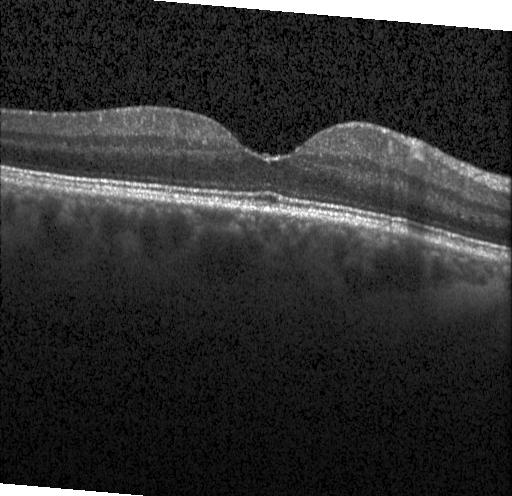 Optical coherence tomography B-scan — Macular OCT: no evidence of choroidal neovascularization, diabetic macular edema, or drusen.